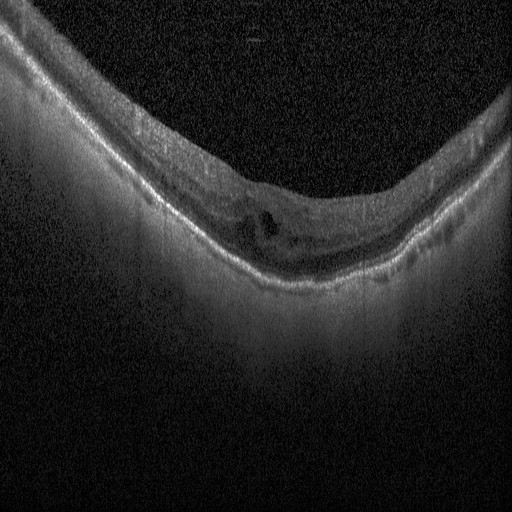
Finding: diabetic macular edema.